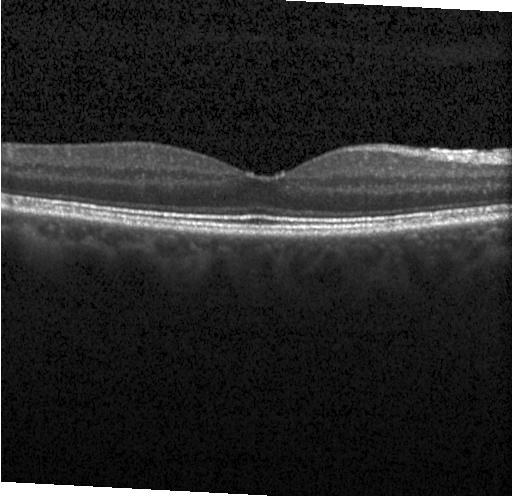 Macular OCT demonstrating no choroidal neovascularization, no diabetic macular edema, and no drusen.